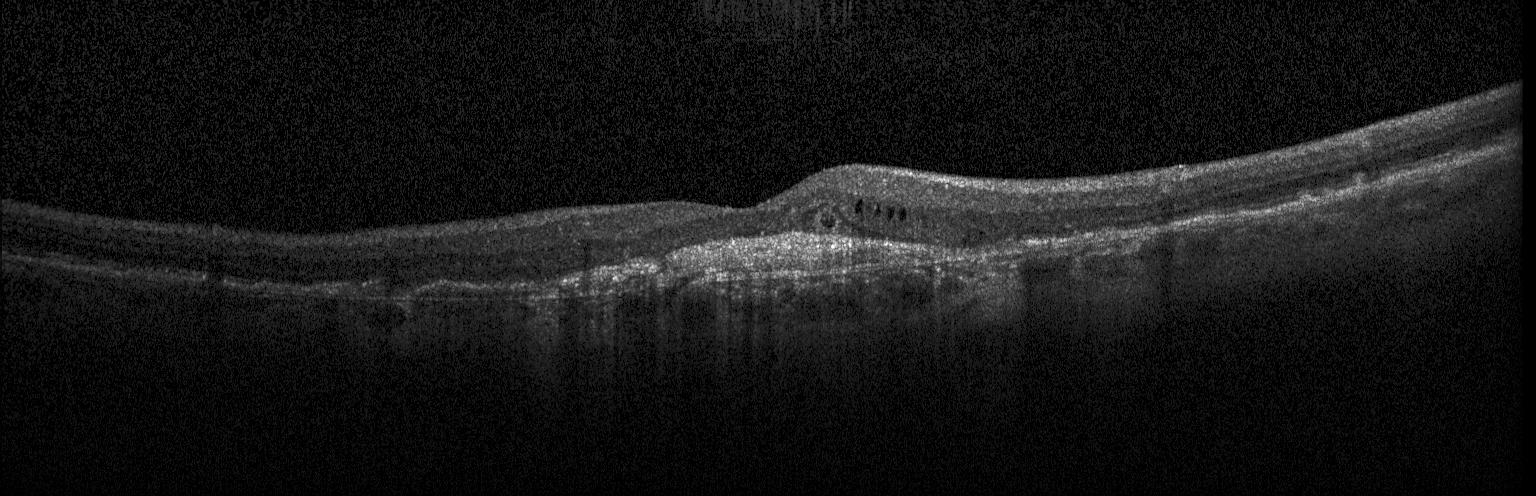

Macular scan · optical coherence tomography scan · instrument: Heidelberg Spectralis.
Diagnosis: a choroidal neovascular membrane.